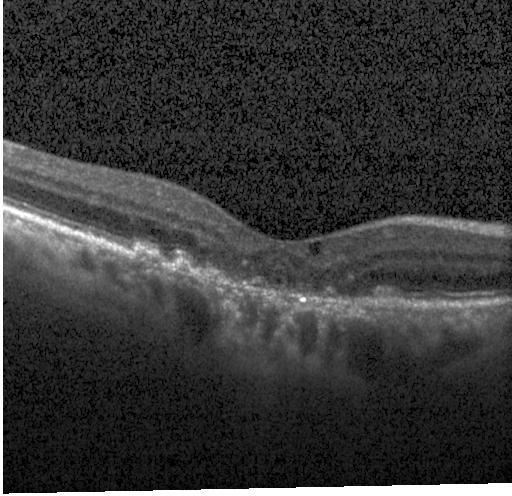 Retinal OCT cross-section. The scan shows choroidal neovascularization (CNV).